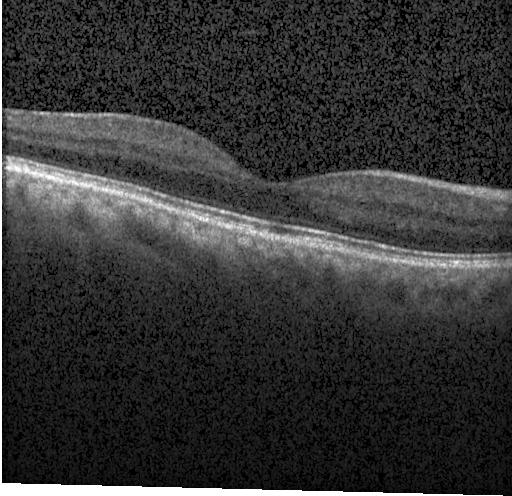 Impression: neither CNV, DME, nor drusen.